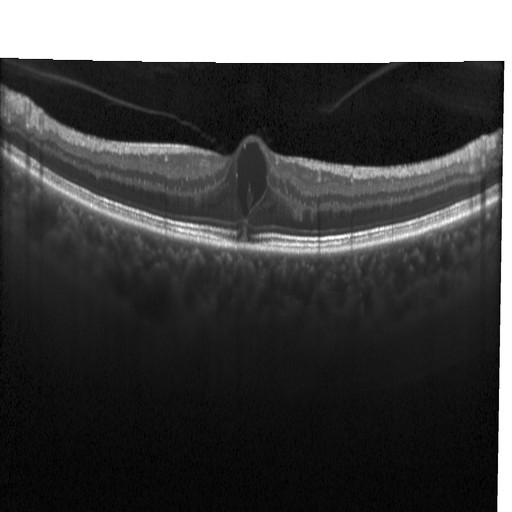

Retinal OCT cross-section; through the macula.
Macular OCT: diabetic macular edema.